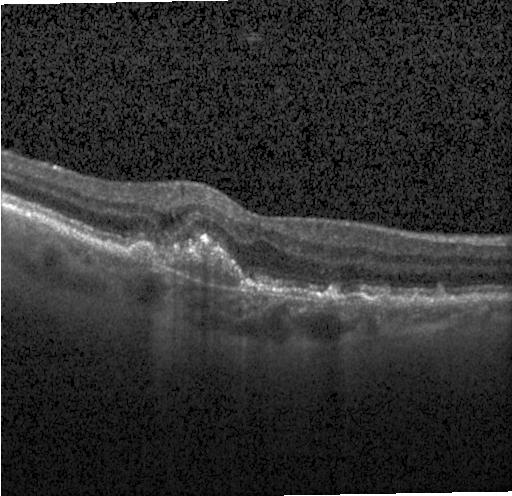

OCT scan showing a choroidal neovascular membrane.